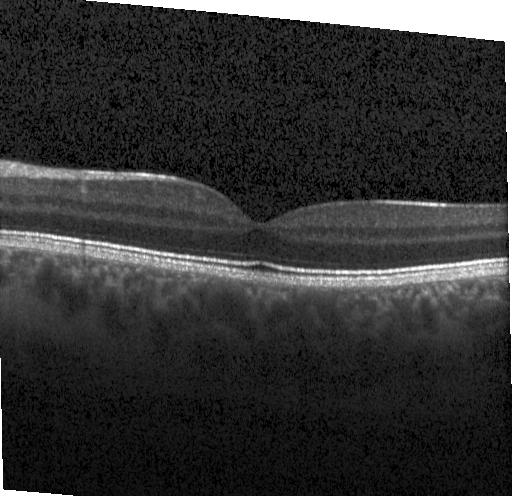
Optical coherence tomography scan
OCT finding: no choroidal neovascularization, diabetic macular edema, or drusen.